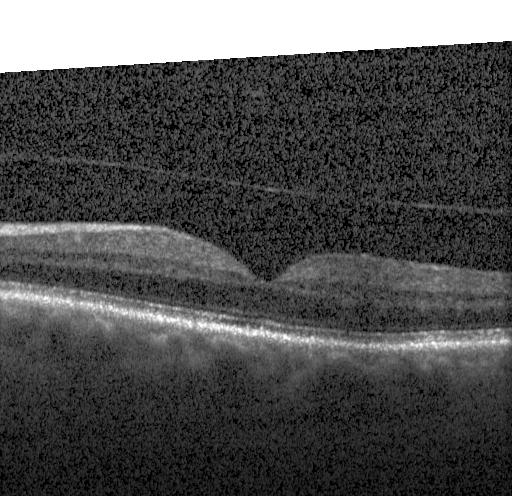
Macular OCT demonstrating no CNV, DME, or drusen.